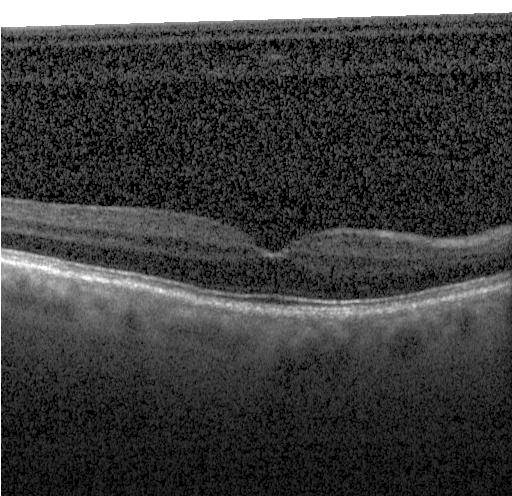
Spectral-domain optical coherence tomography, OCT B-scan
Finding: no choroidal neovascularization, diabetic macular edema, or drusen.